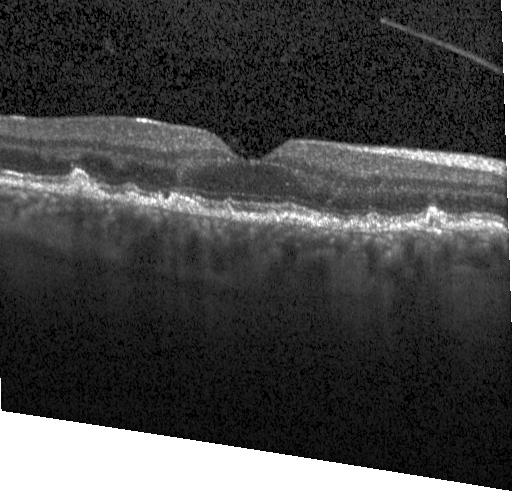
OCT B-scan. Diagnosis: sub-RPE drusenoid deposits.